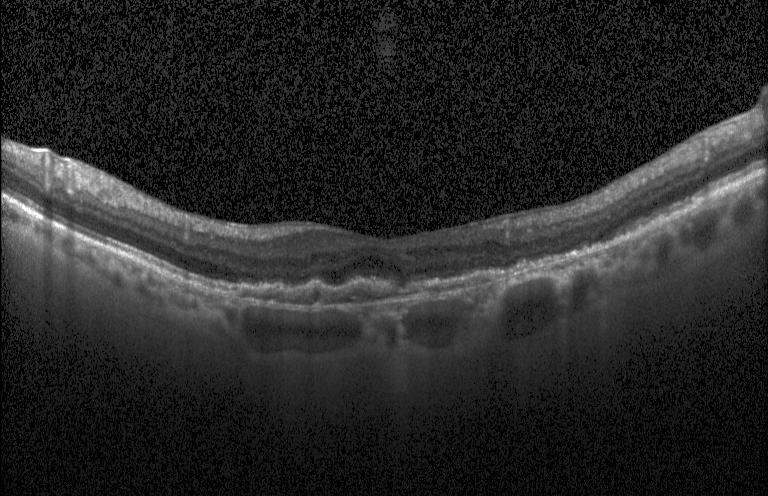
Retinal OCT B-scan — Finding: a choroidal neovascular membrane.